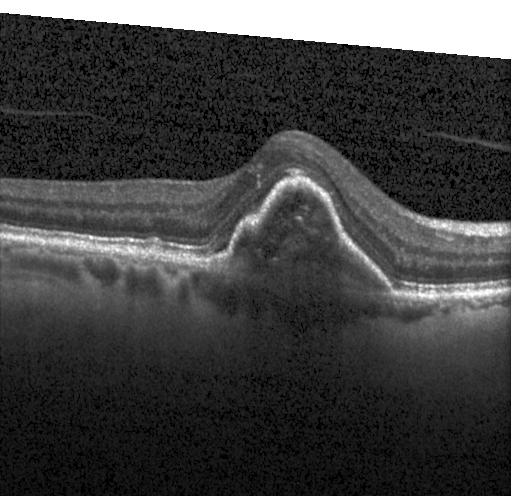
Spectral-domain optical coherence tomography, Heidelberg Spectralis, OCT B-scan — Impression: a choroidal neovascular membrane.